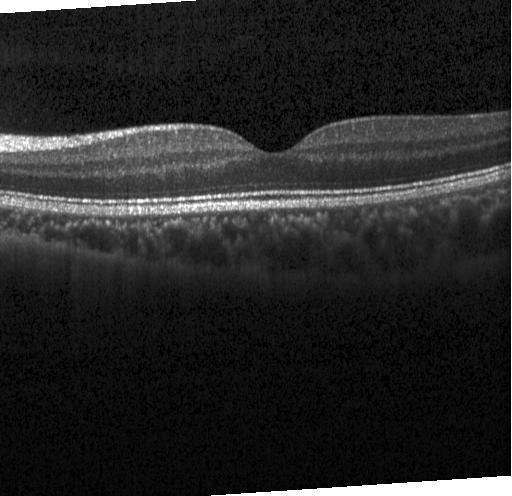

Spectral-domain optical coherence tomography · Heidelberg Spectralis OCT system · OCT line scan — OCT finding: neither choroidal neovascularization, diabetic macular edema, nor drusen.